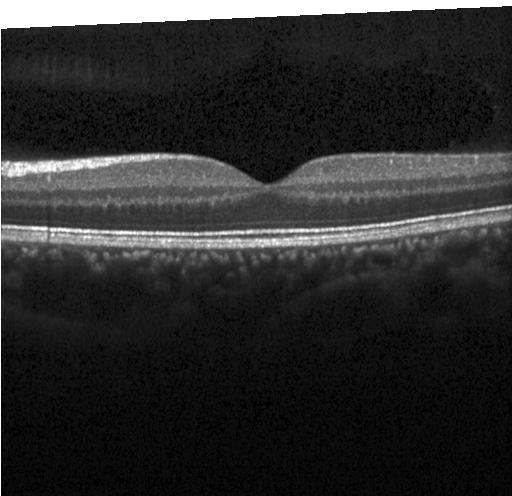 Heidelberg Spectralis OCT system; OCT line scan; spectral-domain OCT
Finding: no choroidal neovascularization, no diabetic macular edema, and no drusen.